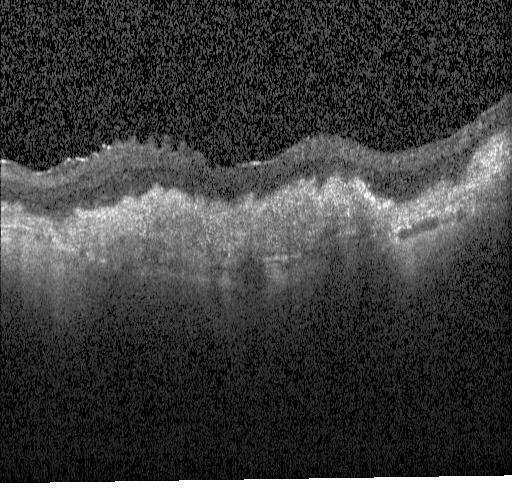

Retinal OCT cross-section. Assessment: a choroidal neovascular membrane.